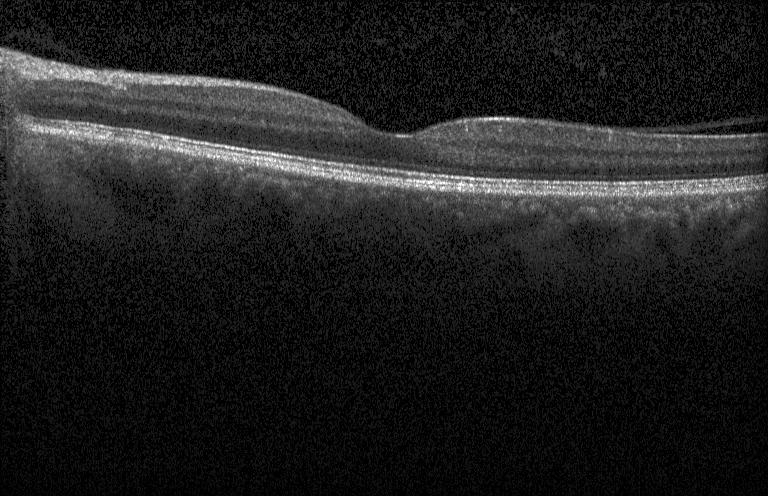 Instrument: Heidelberg Spectralis. SD-OCT. Macular scan. Optical coherence tomography B-scan
Macular OCT: no evidence of CNV, DME, or drusen.